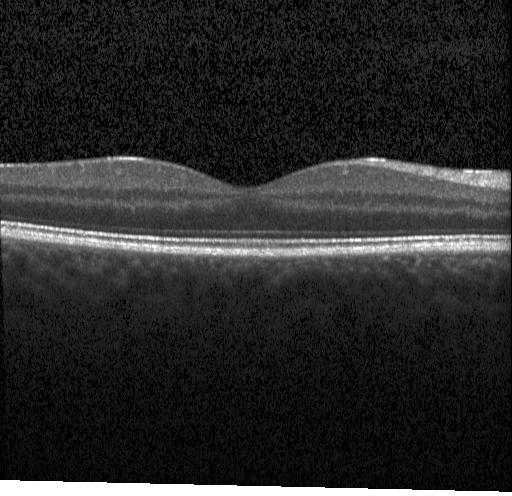 Impression: neither choroidal neovascularization, diabetic macular edema, nor drusen.